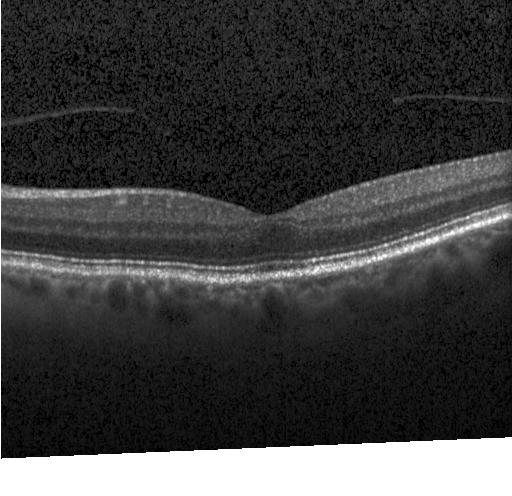
Heidelberg Spectralis OCT system · spectral-domain optical coherence tomography · retinal OCT B-scan.
Assessment: no evidence of choroidal neovascularization, diabetic macular edema, or drusen.